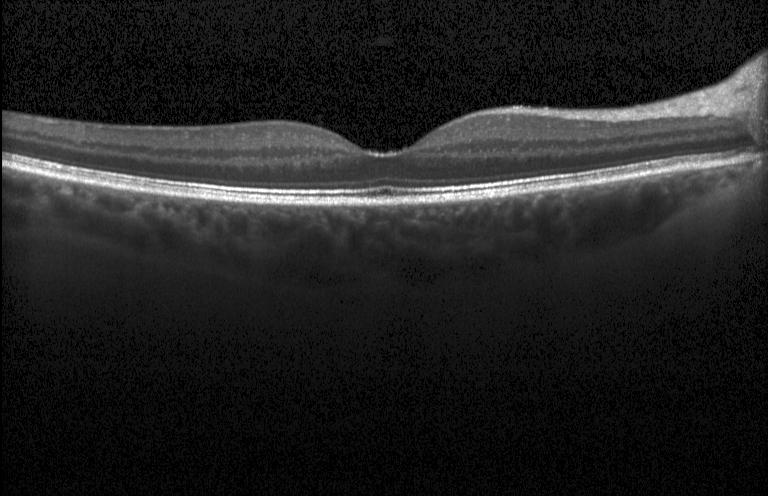
Through the macula; acquired on a Heidelberg Spectralis; optical coherence tomography scan.
Assessment: no CNV, DME, or drusen.